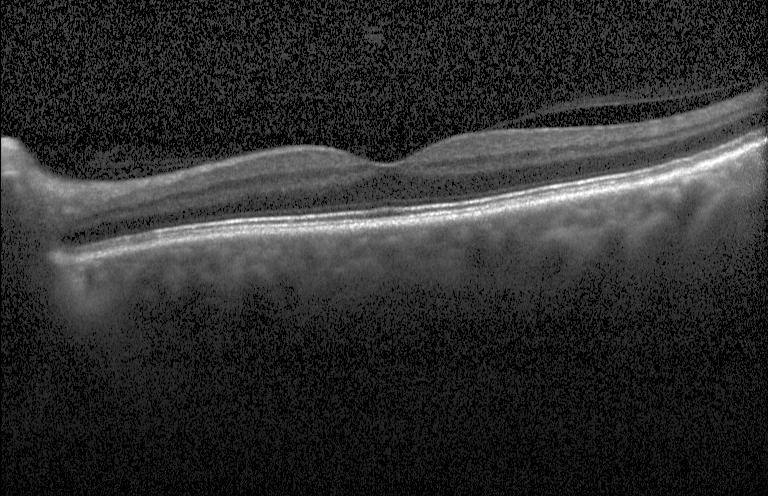

Retinal OCT B-scan. Instrument: Heidelberg Spectralis. Through the macula. SD-OCT. This B-scan demonstrates no choroidal neovascularization, no diabetic macular edema, and no drusen.